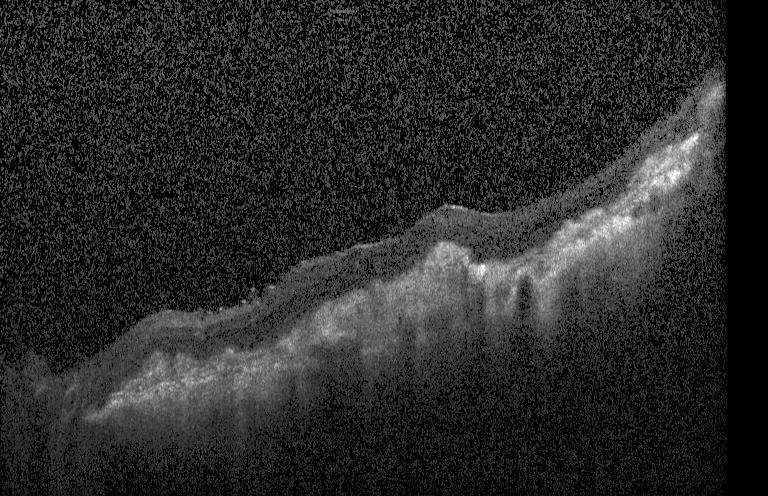 OCT B-scan.
OCT finding: CNV.